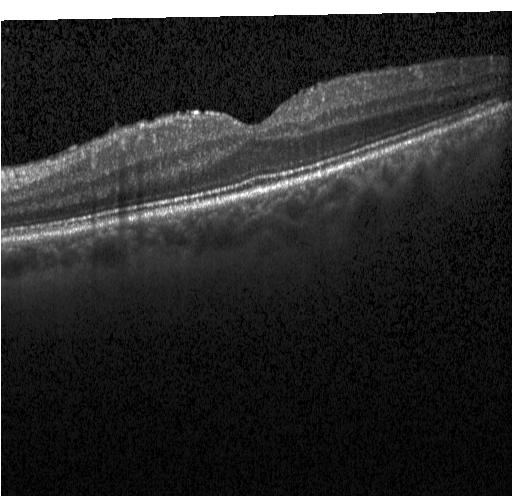
OCT line scan.
This B-scan demonstrates neither choroidal neovascularization, diabetic macular edema, nor drusen.